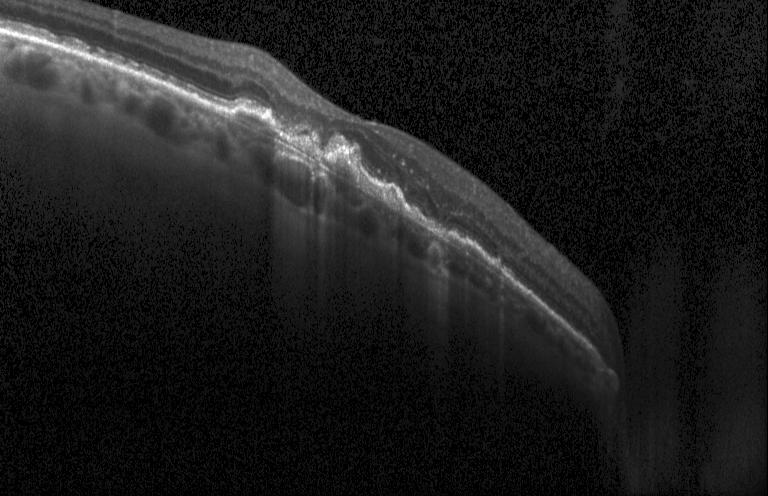
Heidelberg Spectralis, retinal OCT cross-section
This B-scan demonstrates a choroidal neovascular membrane.